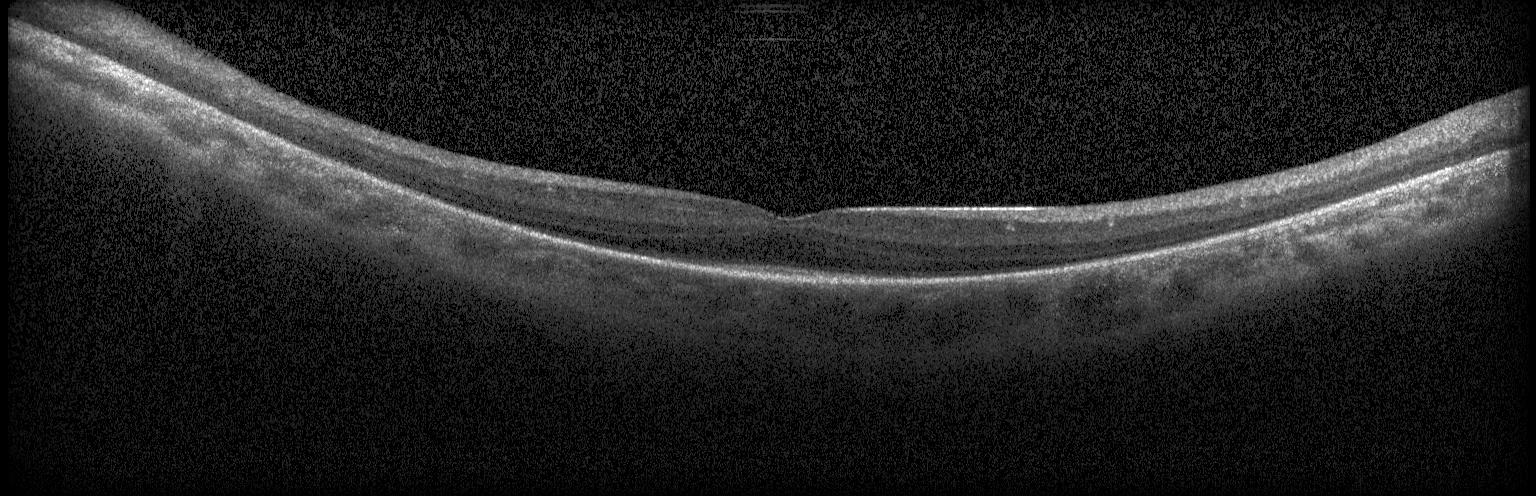 OCT B-scan showing no choroidal neovascularization, no diabetic macular edema, and no drusen.